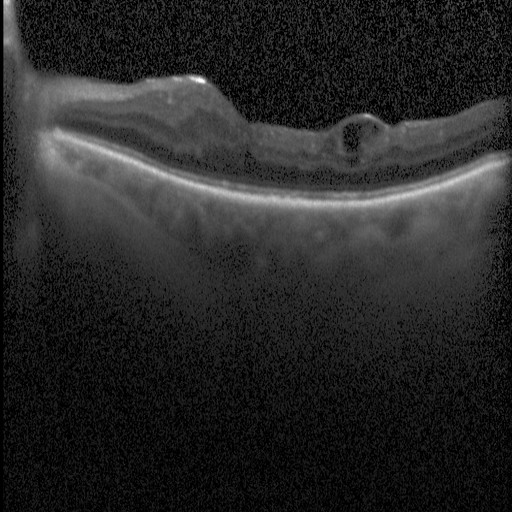 This B-scan demonstrates diabetic macular edema.